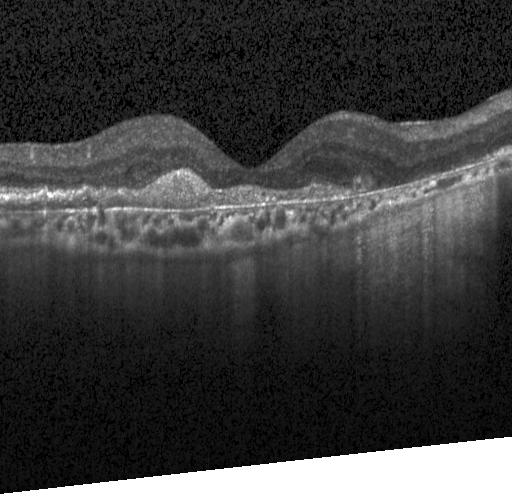
Assessment: choroidal neovascularization.